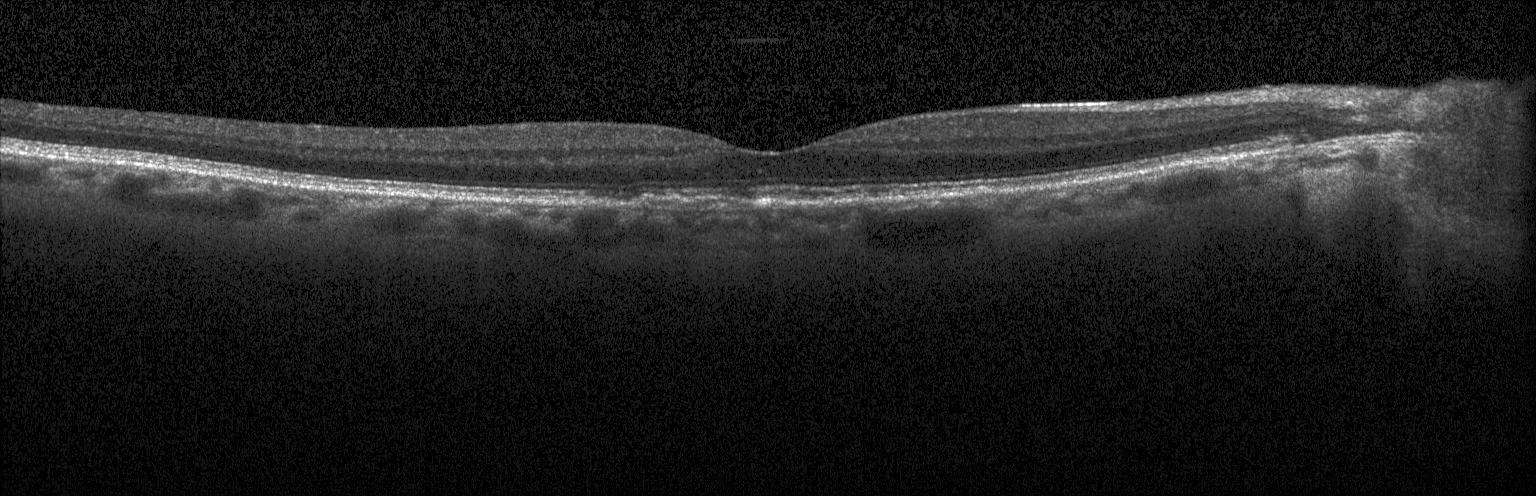
Retinal OCT cross-section.
This B-scan demonstrates sub-RPE drusenoid deposits.